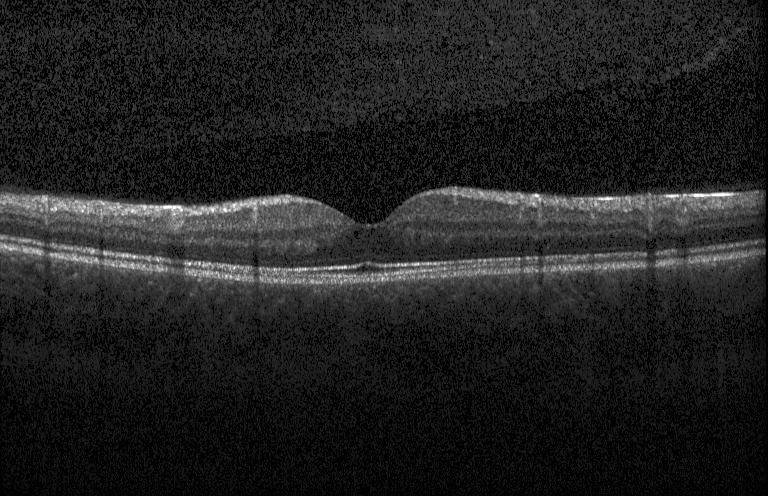
OCT B-scan — Dx: no CNV, DME, or drusen.